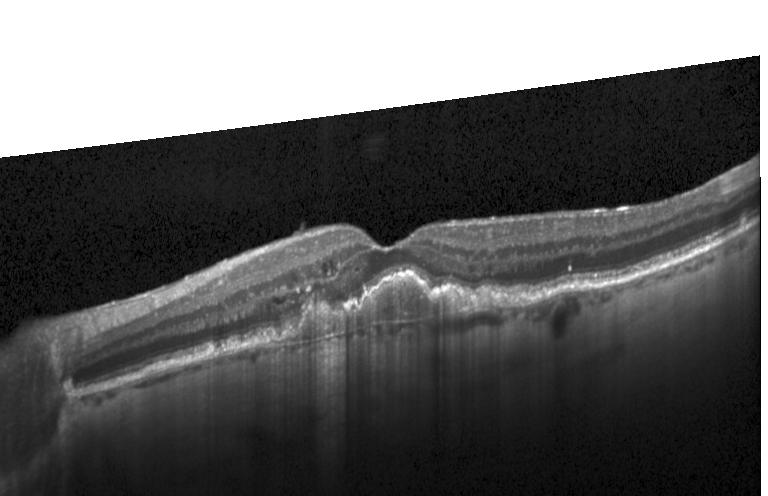

Diagnosis: a choroidal neovascular membrane.